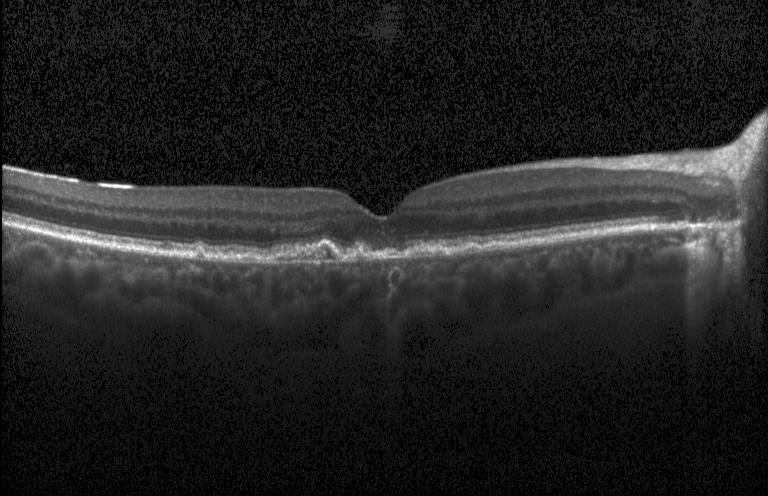 Retinal OCT B-scan; spectral-domain optical coherence tomography. Finding: CNV.